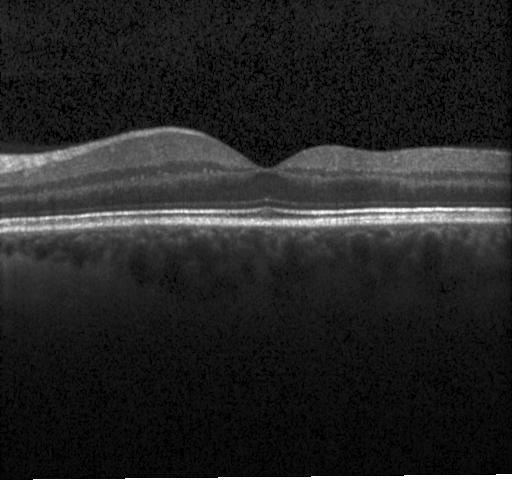 Optical coherence tomography scan. No choroidal neovascularization, diabetic macular edema, or drusen.